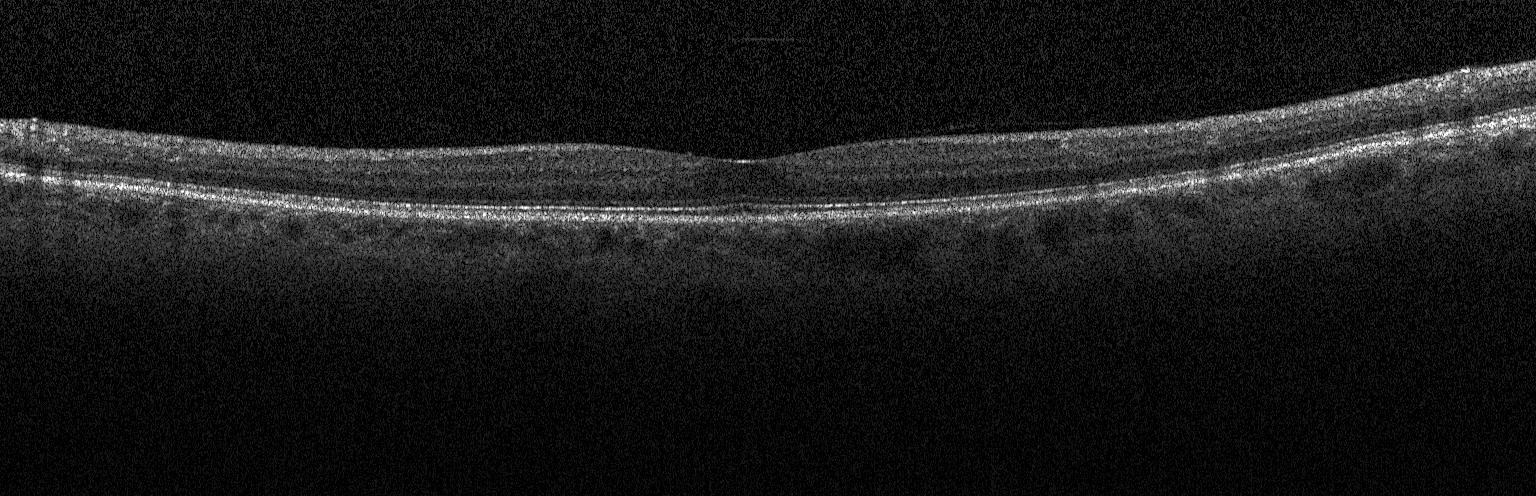
Dx: neither CNV, DME, nor drusen.